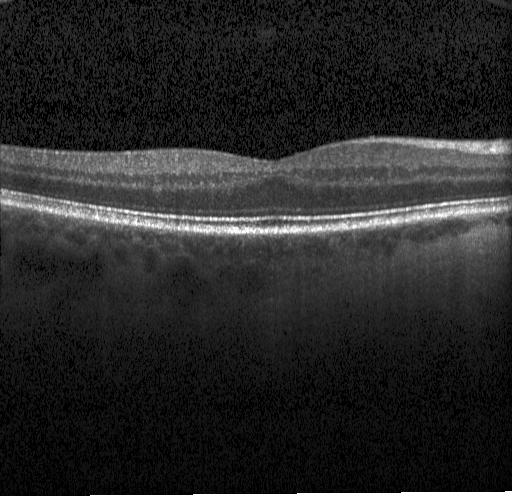 OCT B-scan. Dx: no evidence of CNV, DME, or drusen.